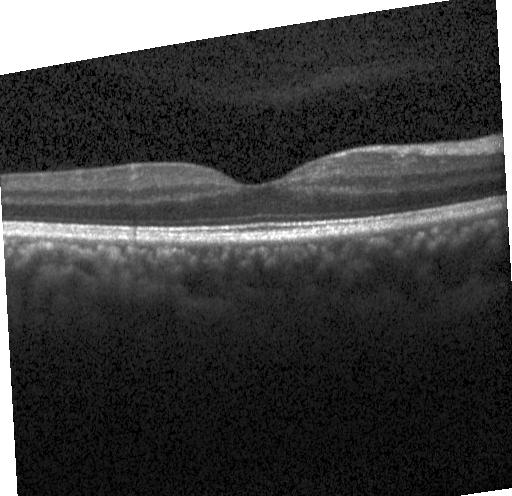
Macular OCT: no CNV, DME, or drusen.